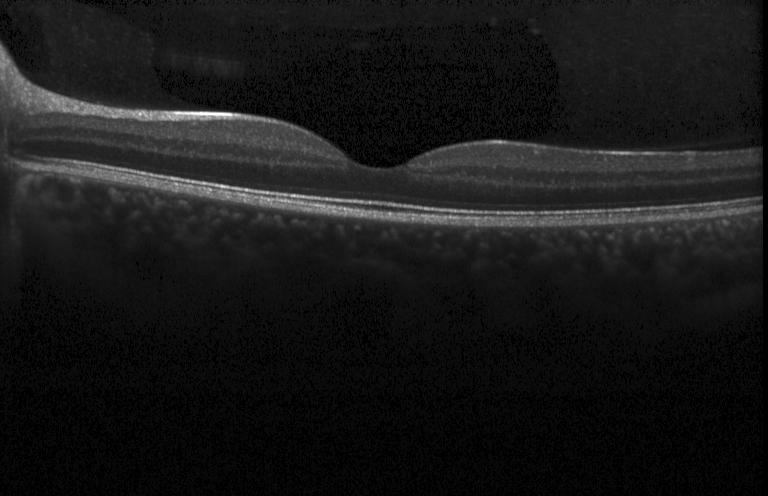

OCT scan showing no choroidal neovascularization, no diabetic macular edema, and no drusen.